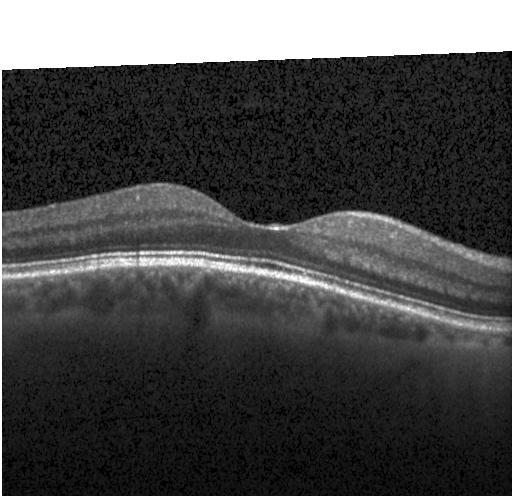

Centered on the fovea; spectral-domain optical coherence tomography; instrument: Heidelberg Spectralis; retinal OCT B-scan — Diagnosis: neither choroidal neovascularization, diabetic macular edema, nor drusen.